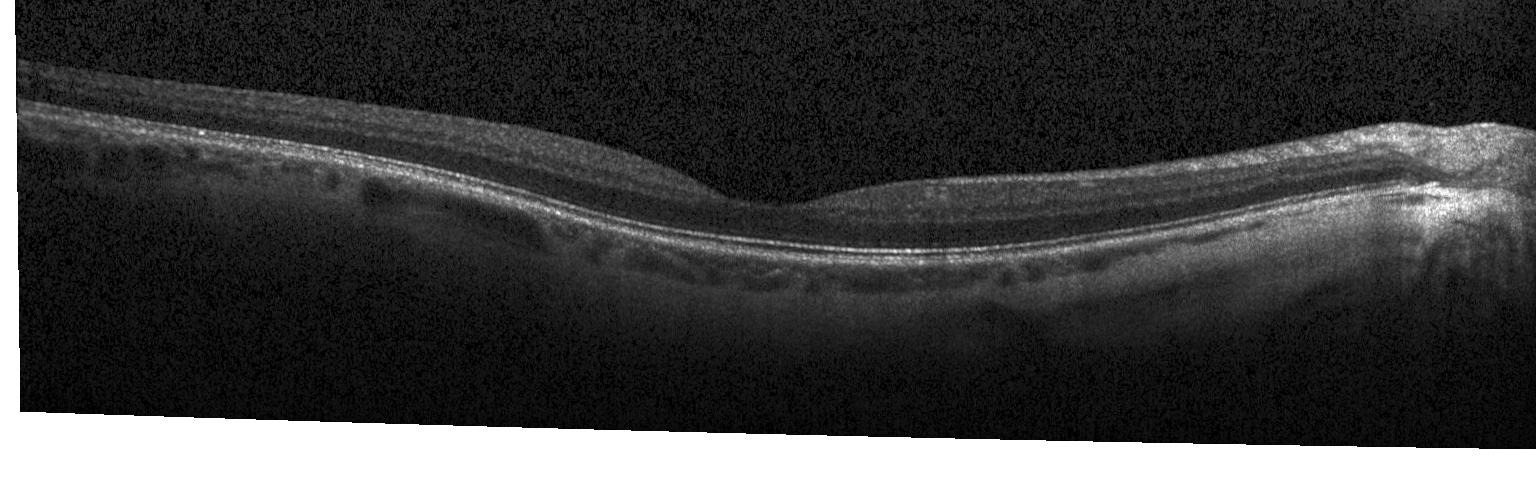 Spectral-domain OCT B-scan: no choroidal neovascularization, diabetic macular edema, or drusen.